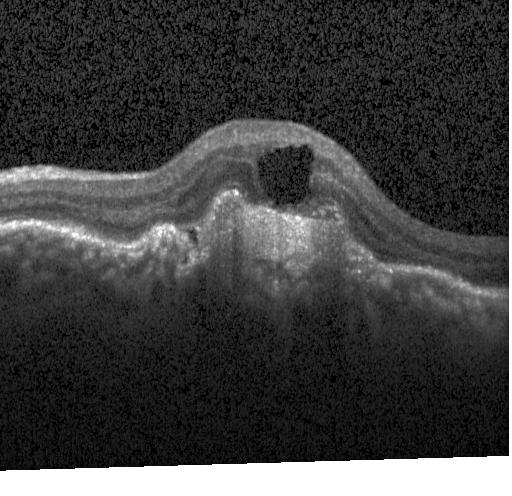
Optical coherence tomography scan.
Impression: a choroidal neovascular membrane.